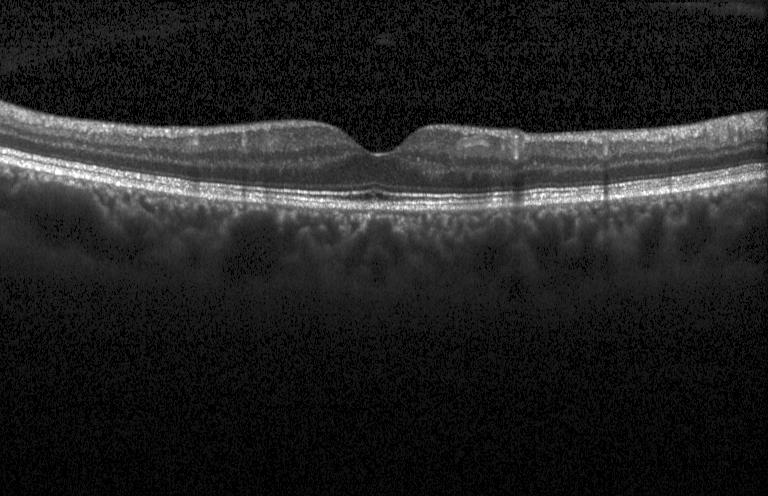
OCT B-scan. Instrument: Heidelberg Spectralis. Assessment: neither choroidal neovascularization, diabetic macular edema, nor drusen.